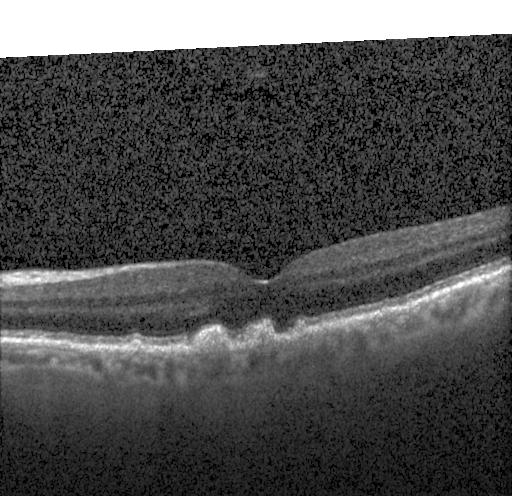
Assessment: multiple drusen.